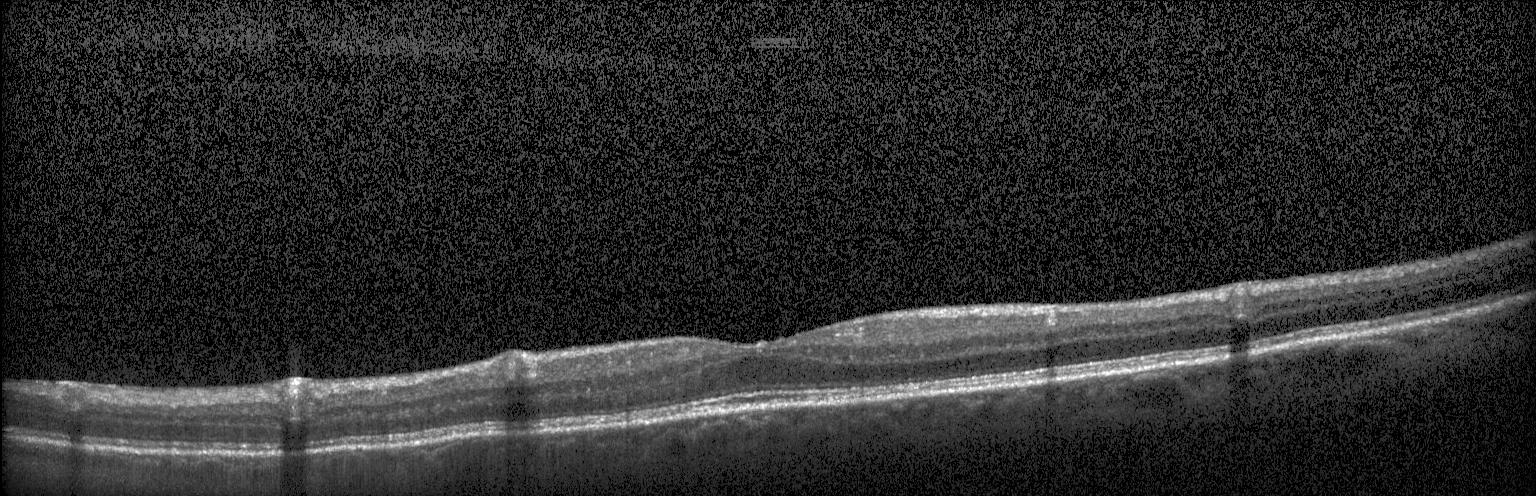 Diagnosis: no choroidal neovascularization, no diabetic macular edema, and no drusen.